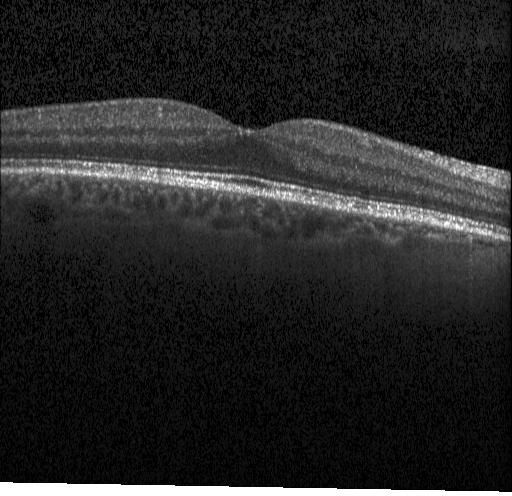 Dx: no CNV, DME, or drusen.